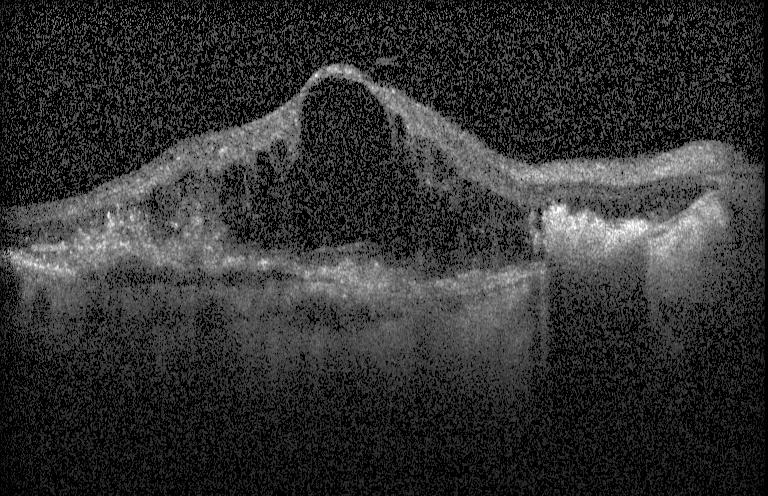
OCT scan showing a choroidal neovascular membrane.